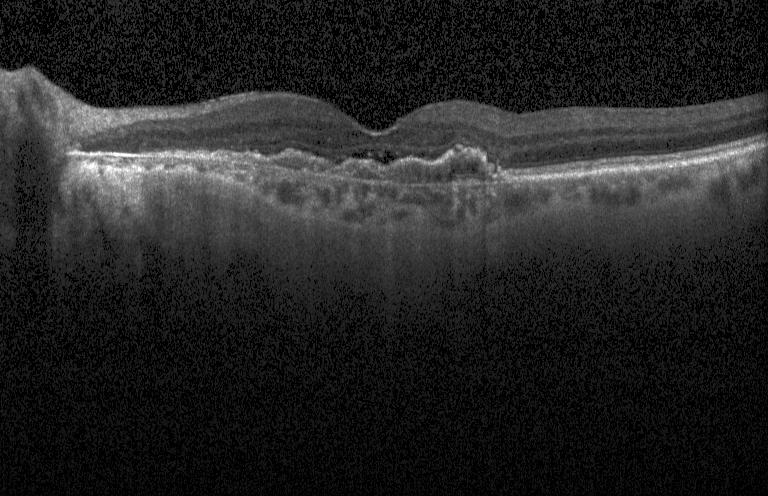

Optical coherence tomography scan, SD-OCT, macular scan — Diagnosis: CNV.